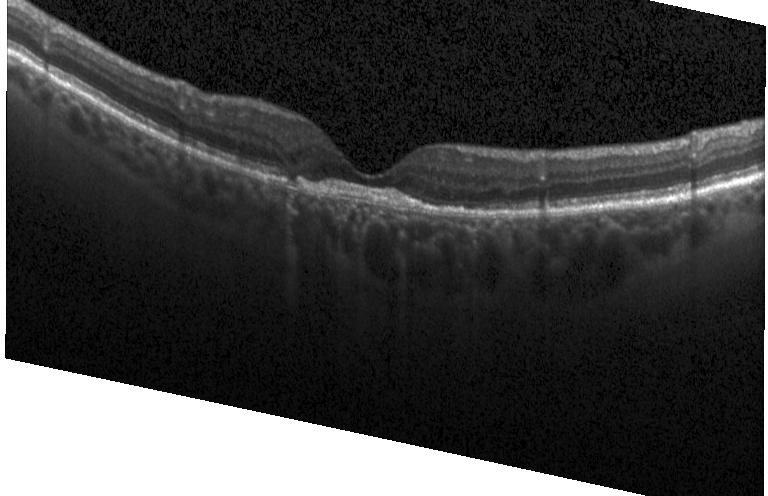 Horizontal scan through the fovea, optical coherence tomography scan.
Impression: choroidal neovascularization (CNV).